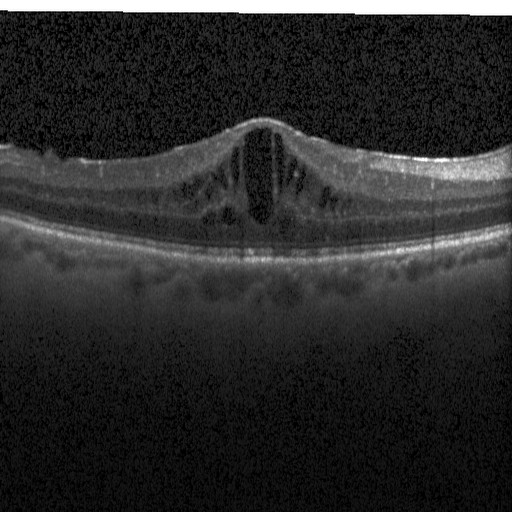 Dx: diabetic macular edema.